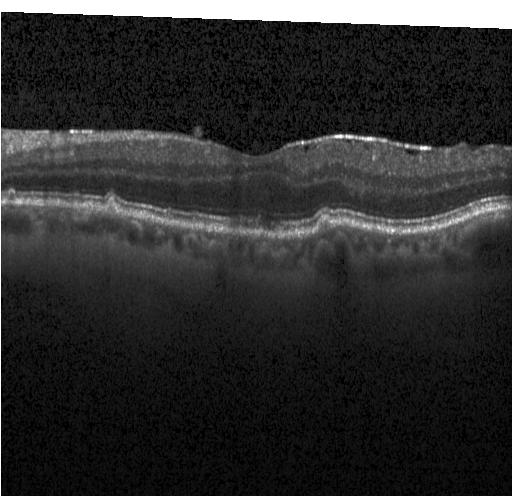 Optical coherence tomography B-scan. This B-scan demonstrates multiple drusen.